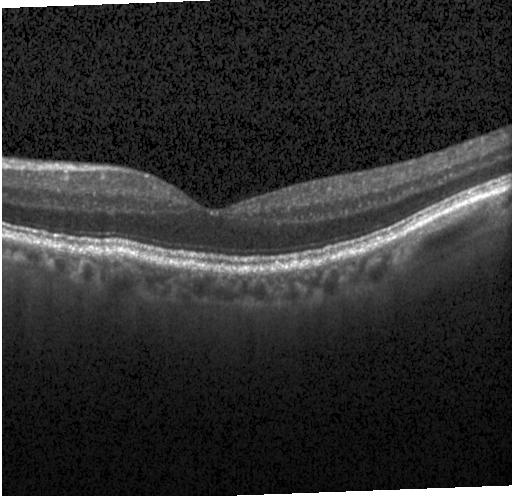

Retinal OCT B-scan · centered on the fovea · spectral-domain OCT. Finding: neither choroidal neovascularization, diabetic macular edema, nor drusen.